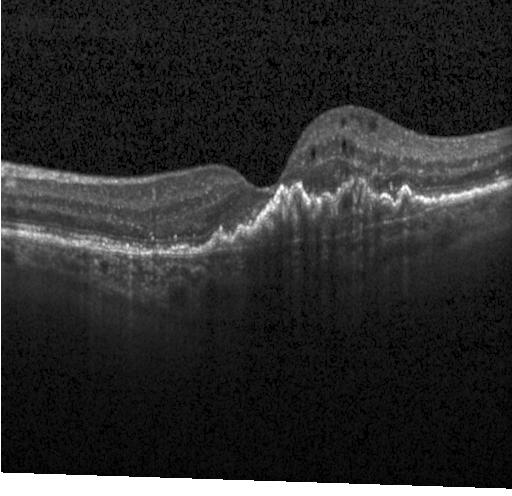 Optical coherence tomography scan
Finding: a choroidal neovascular membrane.